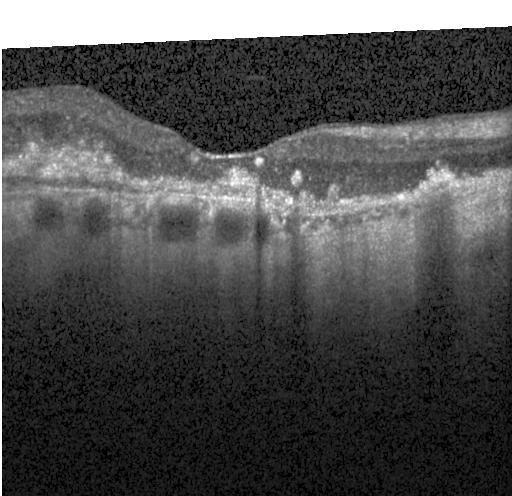
Macular OCT demonstrating choroidal neovascularization.